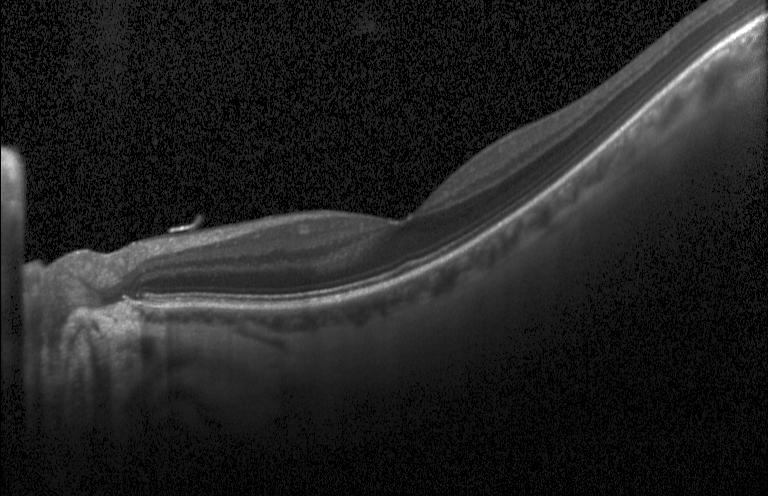 OCT line scan. Through the macula. Finding: no CNV, no DME, and no drusen.